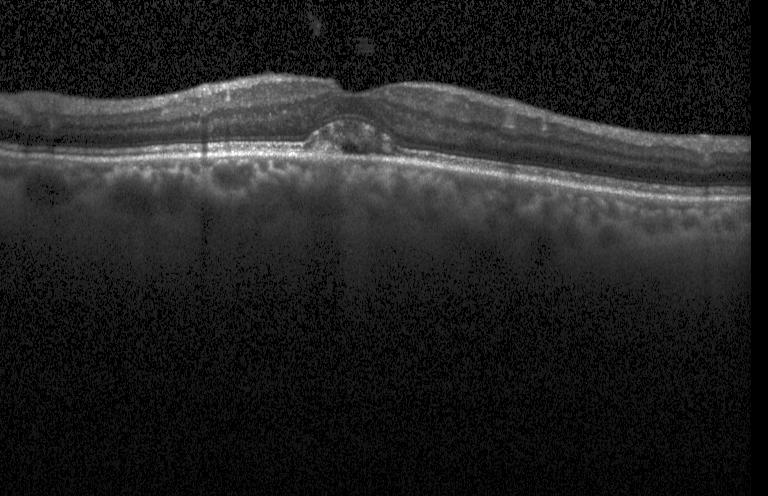

A choroidal neovascular membrane.